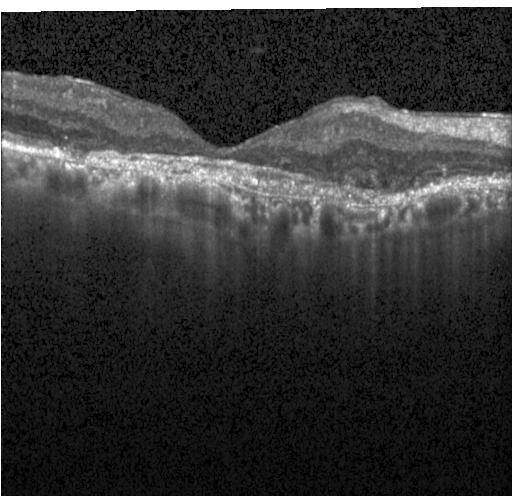 Optical coherence tomography scan. Fovea-centered. Heidelberg Spectralis — Macular OCT: a choroidal neovascular membrane.